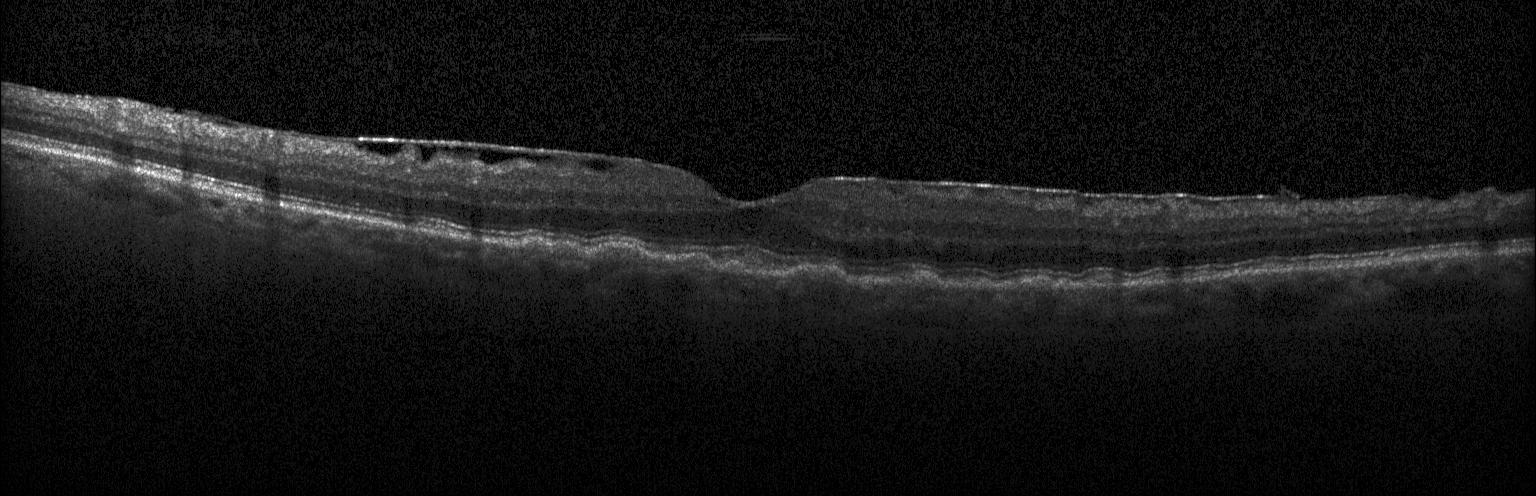

Spectral-domain OCT B-scan: sub-RPE drusenoid deposits.